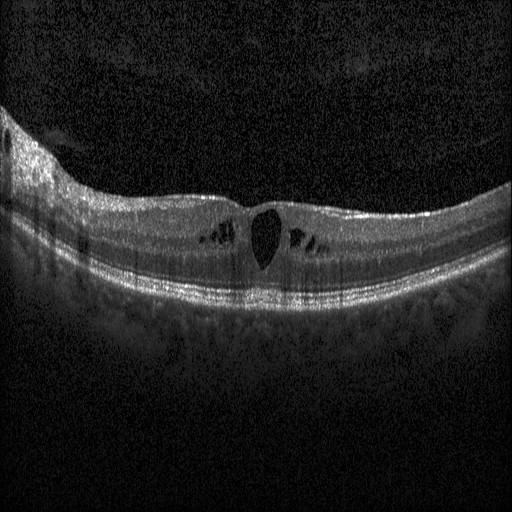 Retinal OCT B-scan; through the macula — Diagnosis: diabetic macular edema (DME).